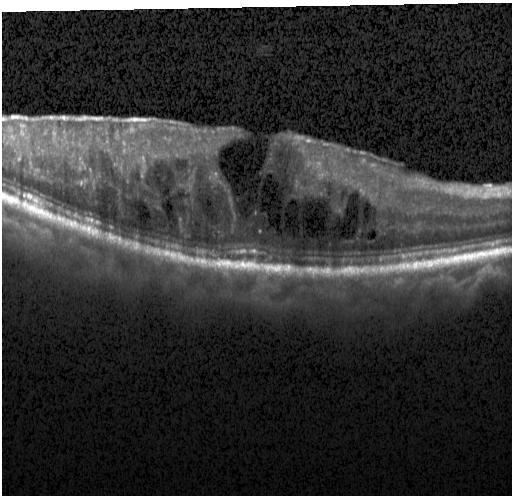 Macular OCT: diabetic macular edema.